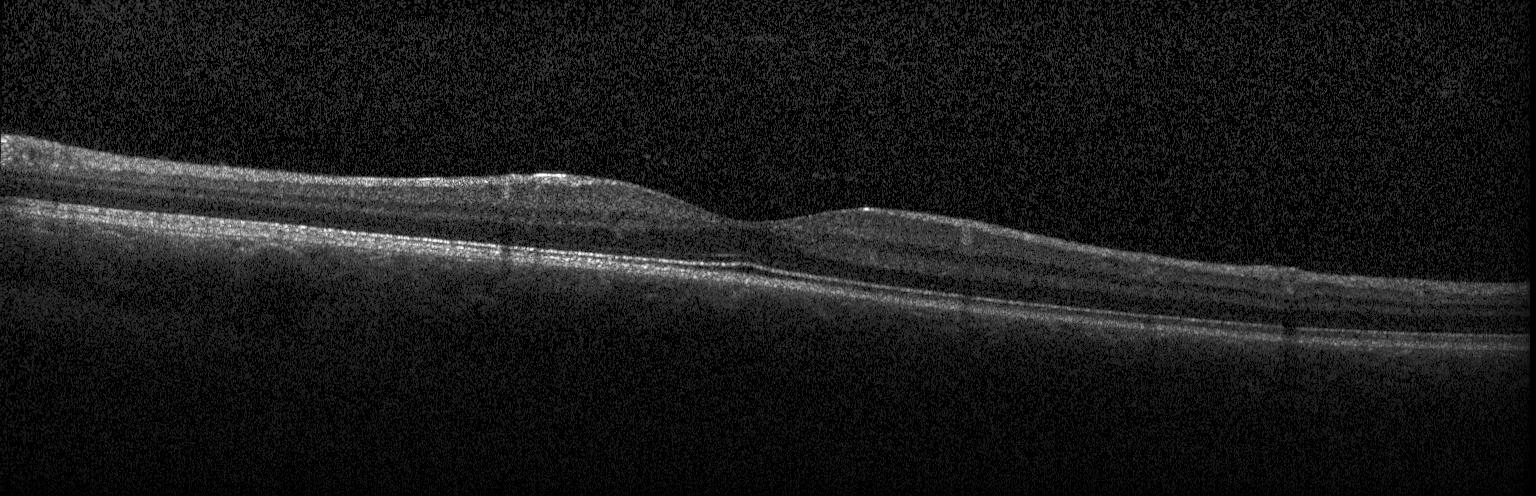

OCT scan showing no CNV, no DME, and no drusen.